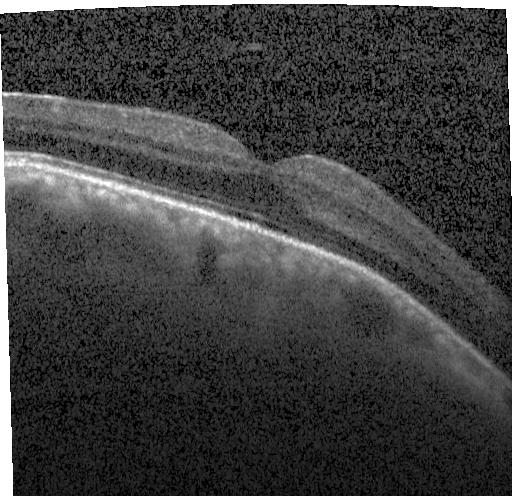

Impression: no choroidal neovascularization, diabetic macular edema, or drusen.